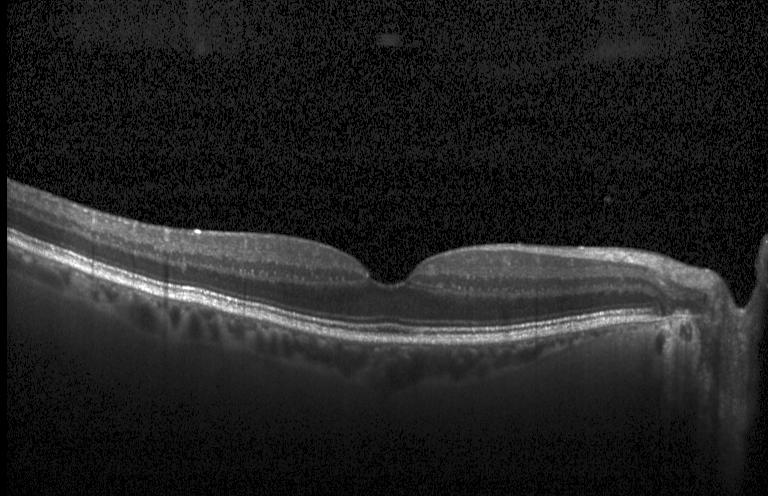

SD-OCT · OCT line scan
Finding: no CNV, DME, or drusen.